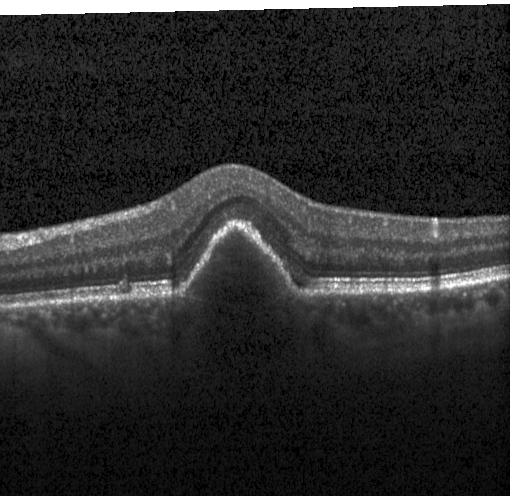
Spectral-domain optical coherence tomography, acquired on a Heidelberg Spectralis, optical coherence tomography B-scan, macular scan. The scan shows choroidal neovascularization.